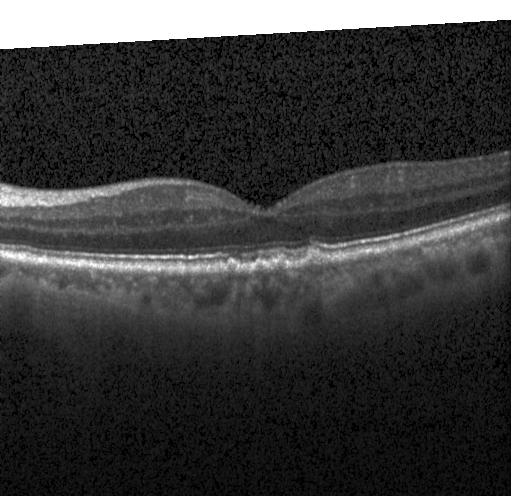 This B-scan demonstrates drusen.